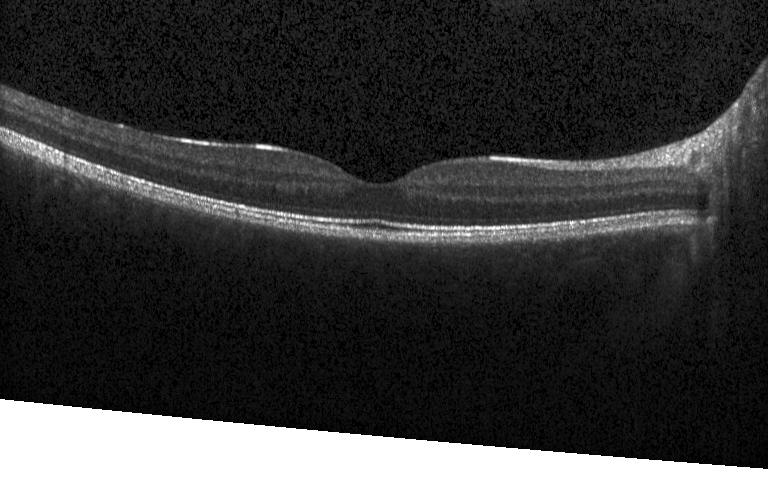 OCT scan showing no evidence of CNV, DME, or drusen.